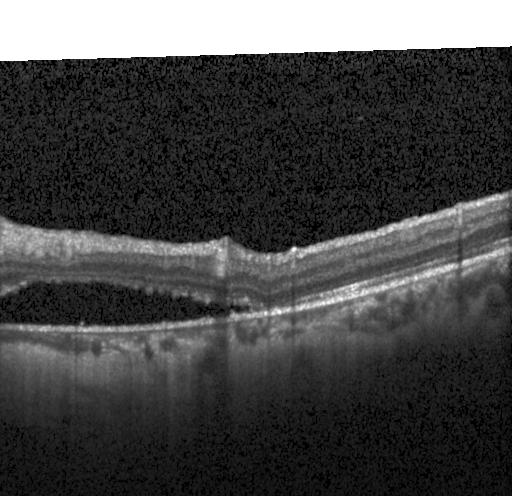
Dx: a choroidal neovascular membrane.